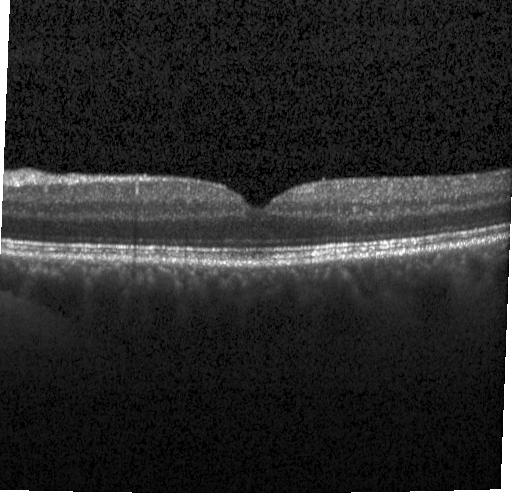

Diagnosis: no CNV, DME, or drusen.